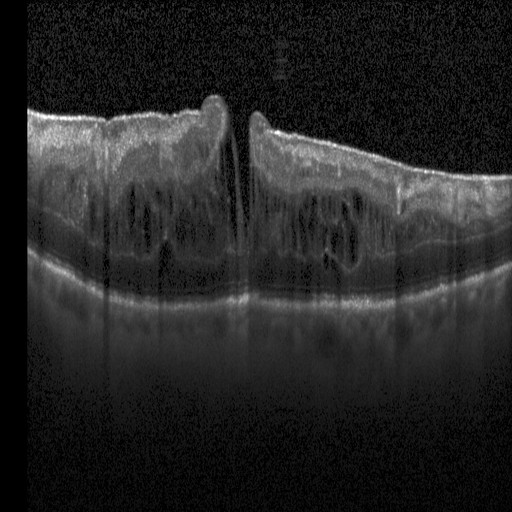
OCT finding: diabetic macular edema (DME).